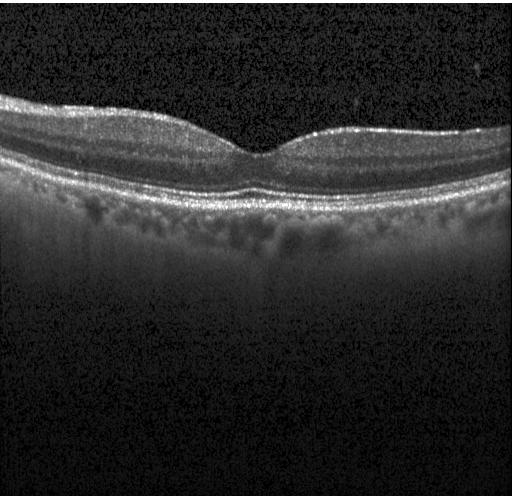
The scan shows no evidence of choroidal neovascularization, diabetic macular edema, or drusen.